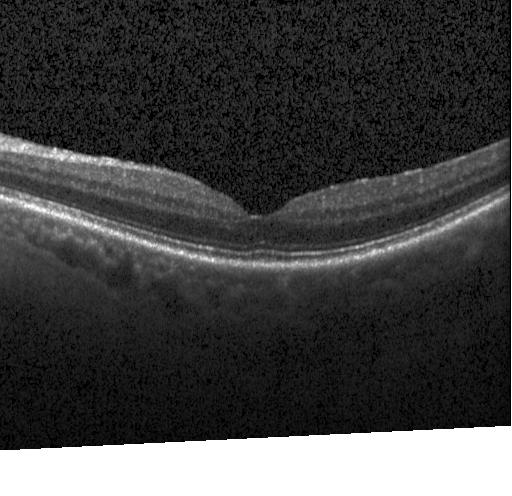
Macular OCT demonstrating no CNV, DME, or drusen.